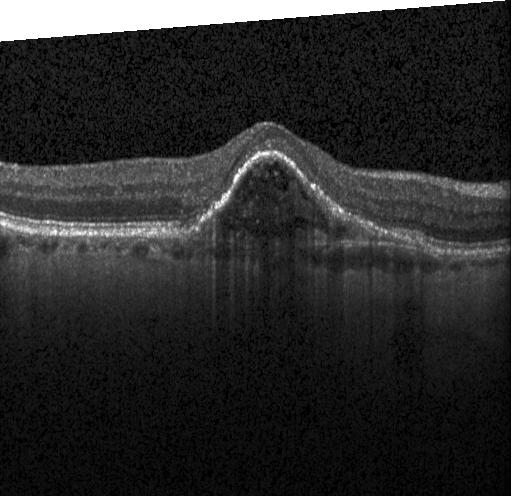 Through the macula, OCT line scan, Heidelberg Spectralis OCT system
Impression: choroidal neovascularization.